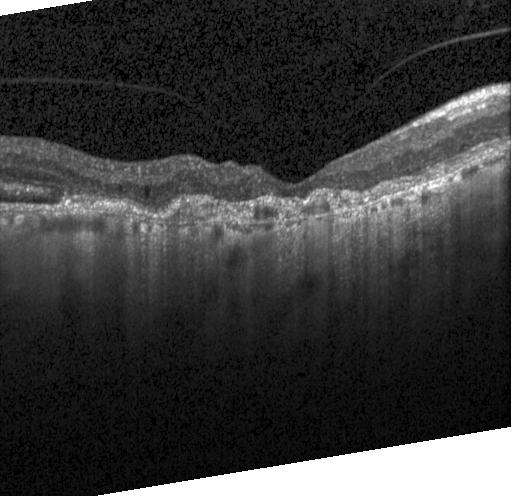
Spectral-domain OCT. Optical coherence tomography scan. Macular scan — A choroidal neovascular membrane.